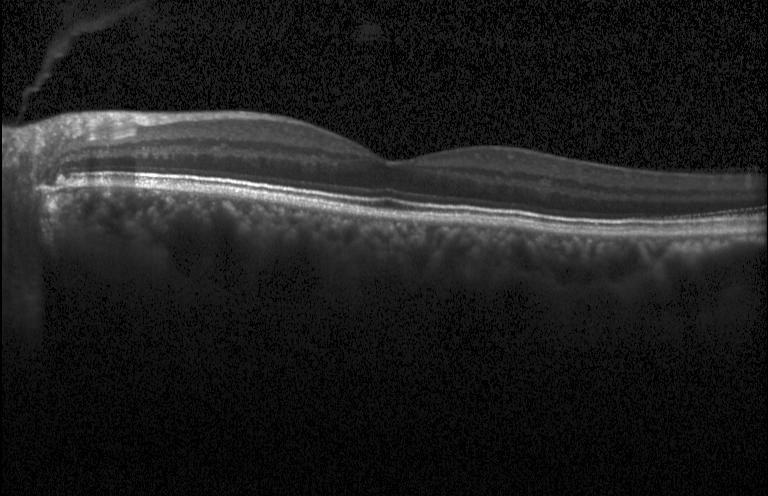

Impression: no choroidal neovascularization, diabetic macular edema, or drusen.